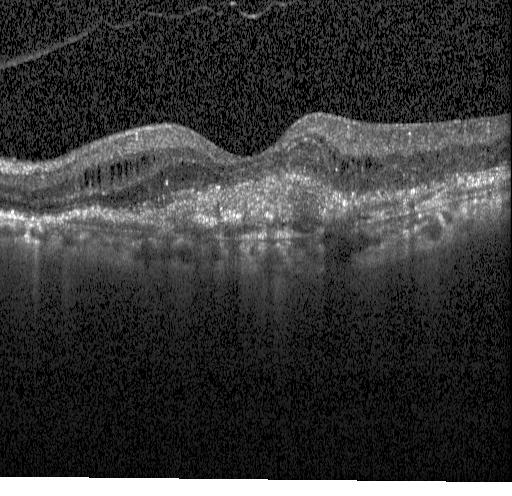 Macular OCT: choroidal neovascularization.